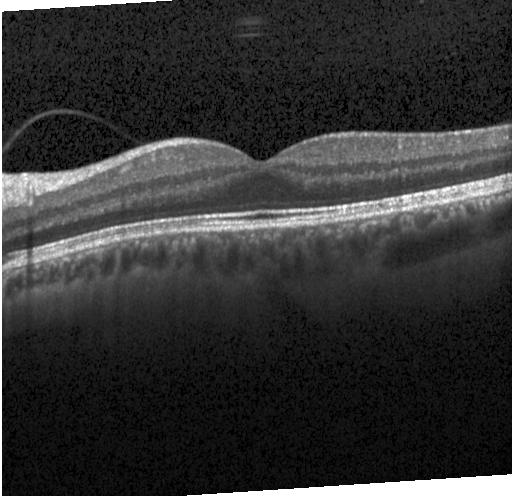 Diagnosis: no choroidal neovascularization, diabetic macular edema, or drusen.